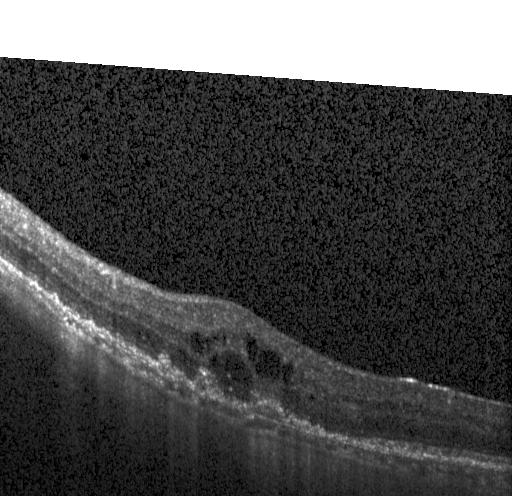

Impression: choroidal neovascularization.